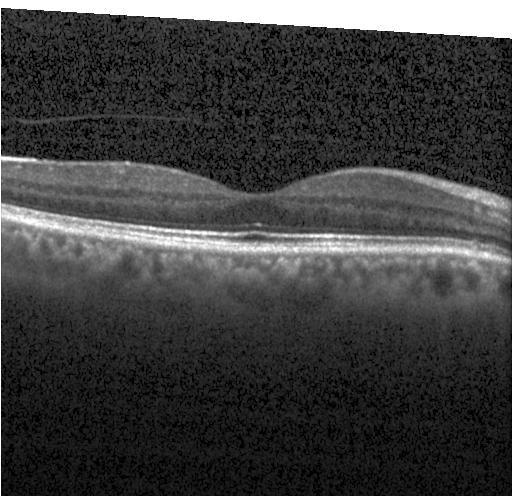
Finding: no choroidal neovascularization, diabetic macular edema, or drusen.